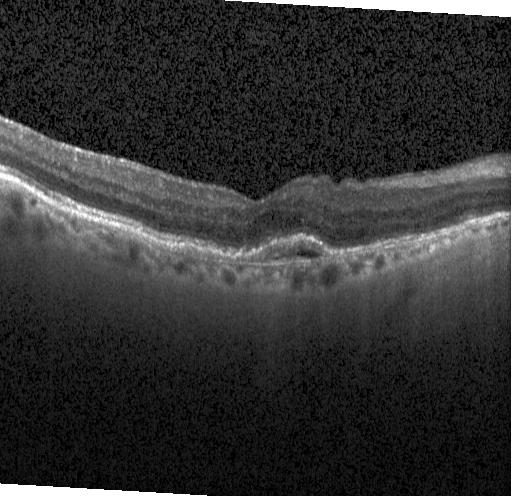 Retinal OCT B-scan. Finding: choroidal neovascularization (CNV).